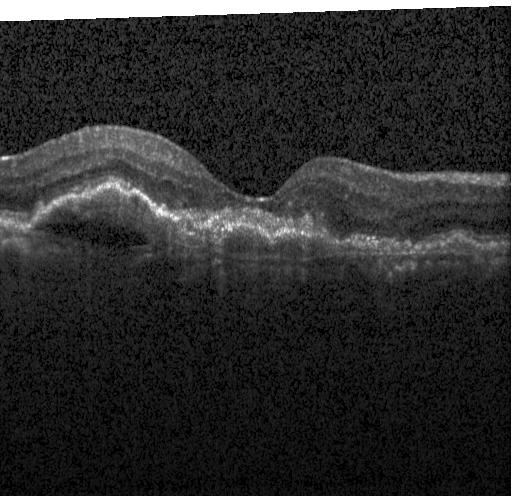 OCT scan showing a choroidal neovascular membrane.